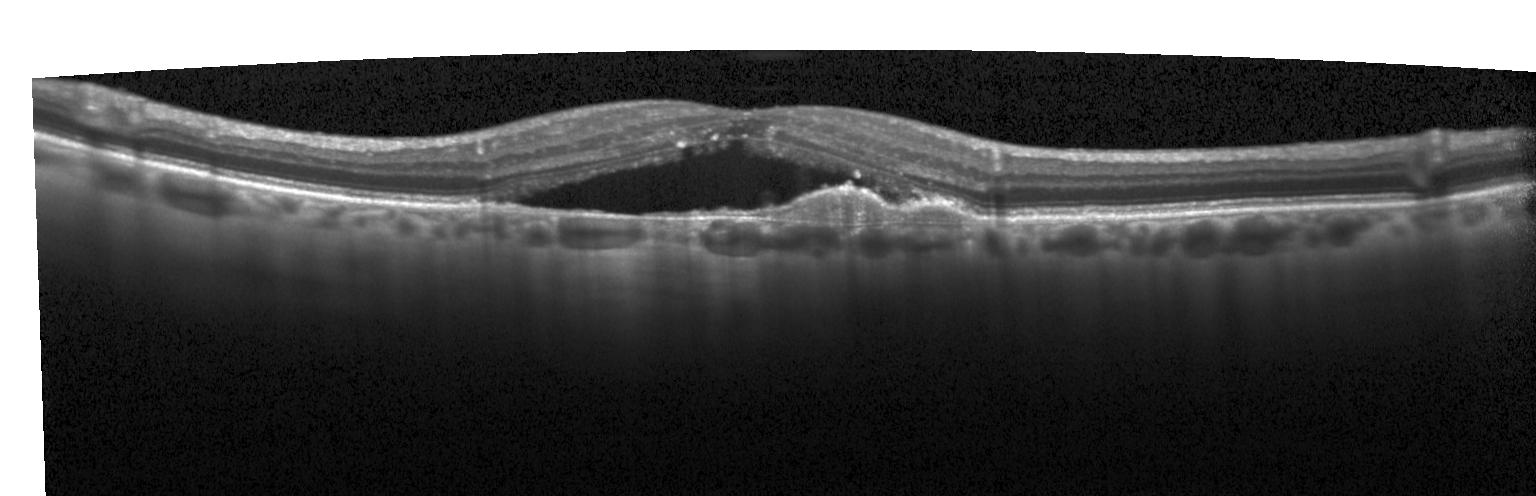 OCT line scan
Finding: a choroidal neovascular membrane.